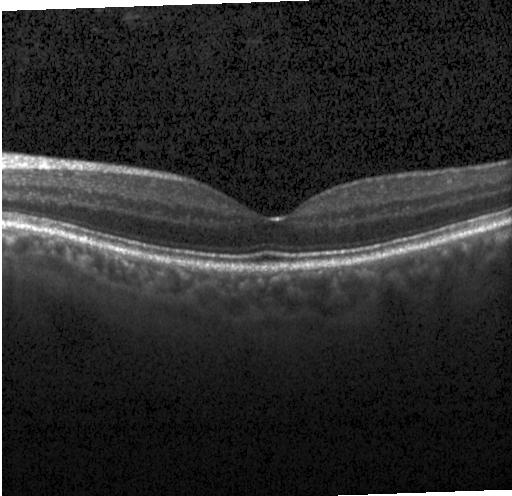
OCT line scan. The scan shows no choroidal neovascularization, diabetic macular edema, or drusen.